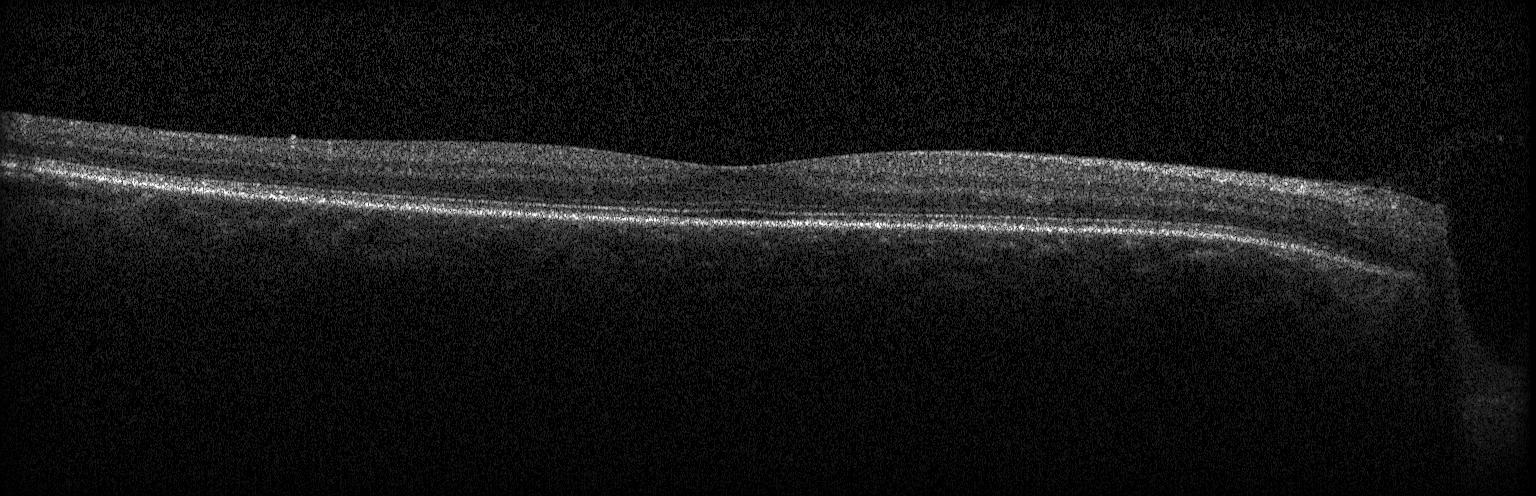 Centered on the fovea, OCT B-scan, Heidelberg Spectralis. Diagnosis: no choroidal neovascularization, diabetic macular edema, or drusen.